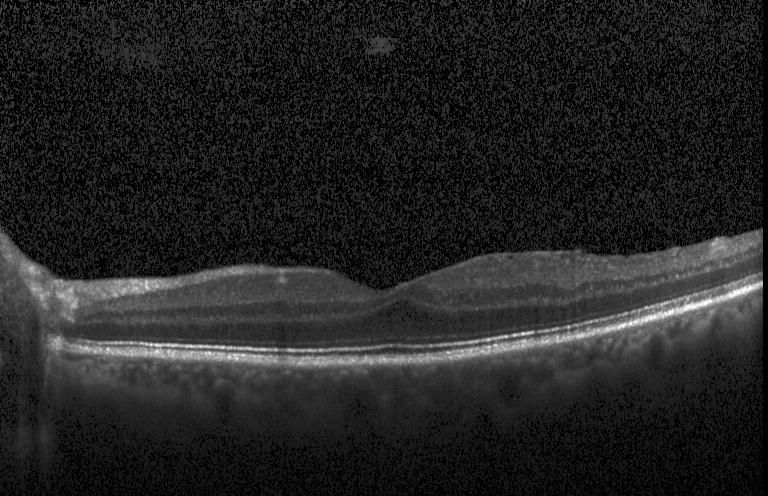 Instrument: Heidelberg Spectralis, OCT B-scan.
Macular OCT: no evidence of choroidal neovascularization, diabetic macular edema, or drusen.